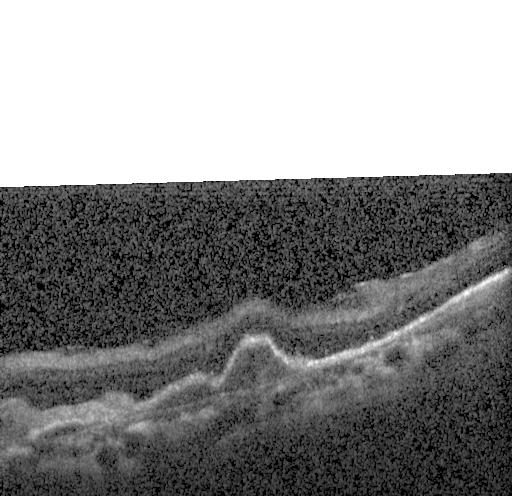
Optical coherence tomography B-scan. Heidelberg Spectralis OCT system. Spectral-domain OCT — Dx: a choroidal neovascular membrane.